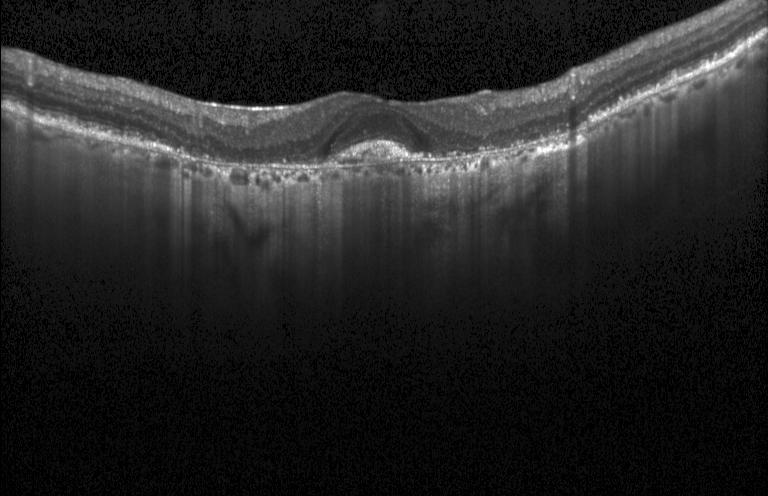

Assessment: choroidal neovascularization (CNV).